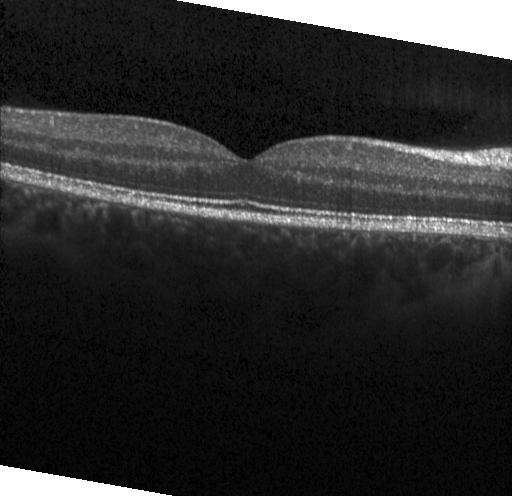 Retinal OCT cross-section. Horizontal scan through the fovea. SD-OCT. Diagnosis: neither choroidal neovascularization, diabetic macular edema, nor drusen.